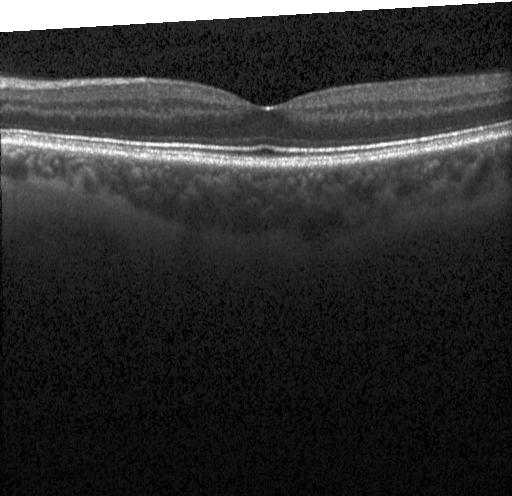
Heidelberg Spectralis OCT system. Spectral-domain optical coherence tomography. Retinal OCT B-scan. Through the macula. Impression: neither CNV, DME, nor drusen.